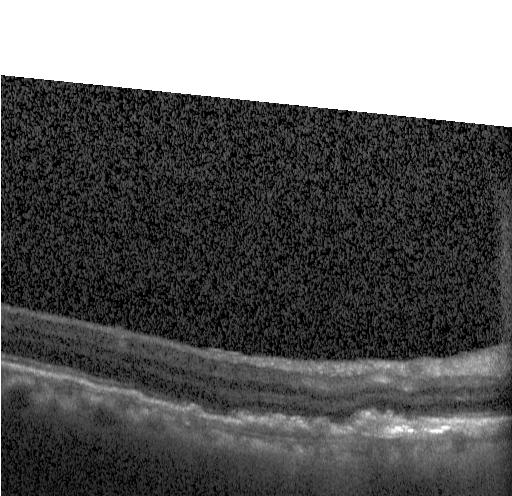

Fovea-centered. Heidelberg Spectralis. Optical coherence tomography scan. SD-OCT
The scan shows CNV.